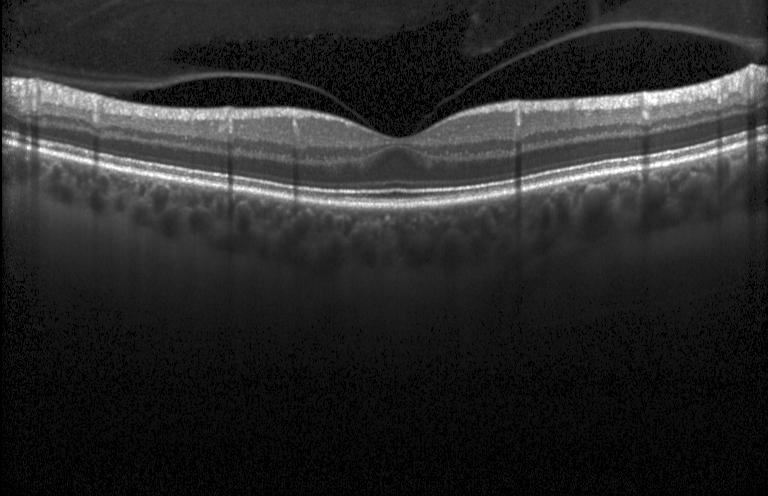
OCT B-scan; centered on the fovea; Heidelberg Spectralis OCT system; spectral-domain OCT
No choroidal neovascularization, no diabetic macular edema, and no drusen.